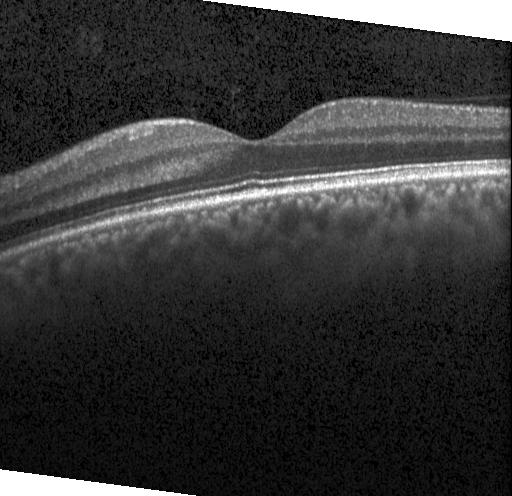 Acquired on a Heidelberg Spectralis; OCT line scan
The scan shows no evidence of choroidal neovascularization, diabetic macular edema, or drusen.